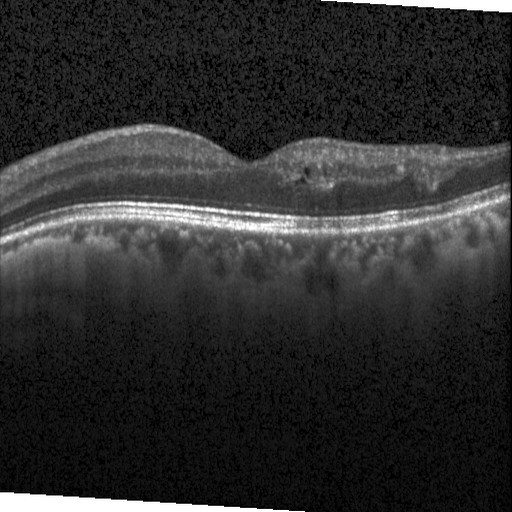

OCT B-scan.
OCT finding: diabetic macular edema.